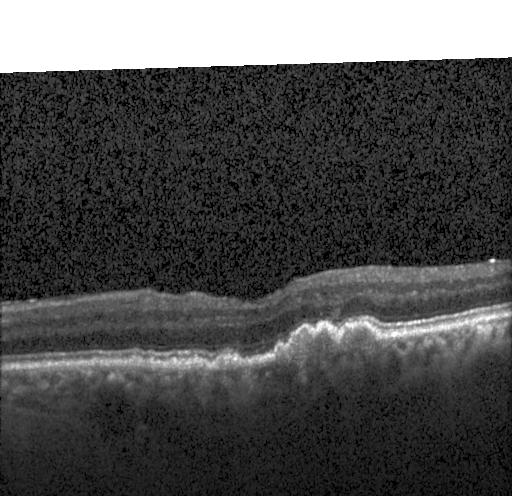

Retinal OCT cross-section showing sub-RPE drusenoid deposits.